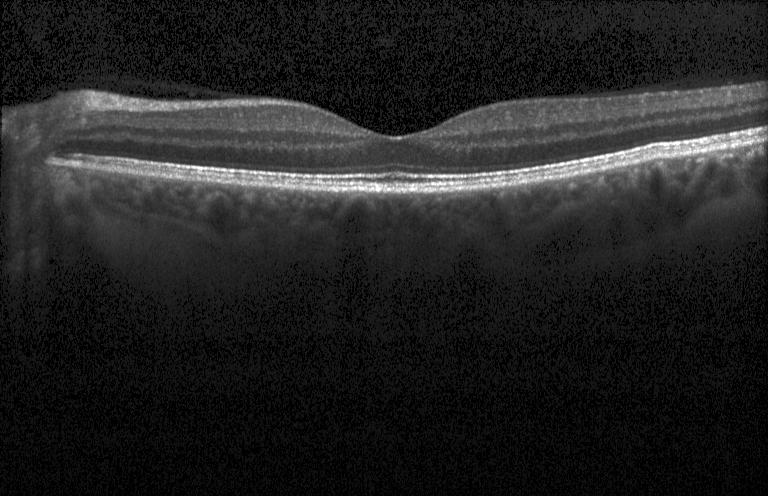

Spectral-domain OCT B-scan: no choroidal neovascularization, no diabetic macular edema, and no drusen.